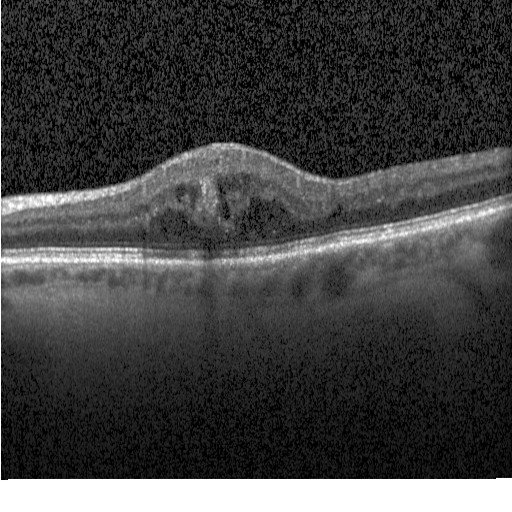 Retinal OCT B-scan — Impression: diabetic macular edema.